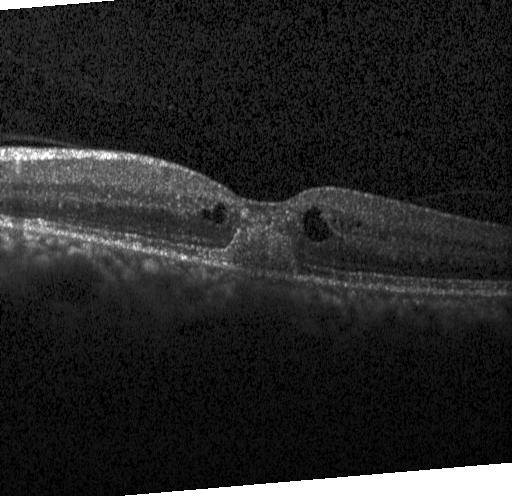 Fovea-centered · optical coherence tomography scan · Heidelberg Spectralis OCT system.
Impression: choroidal neovascularization.